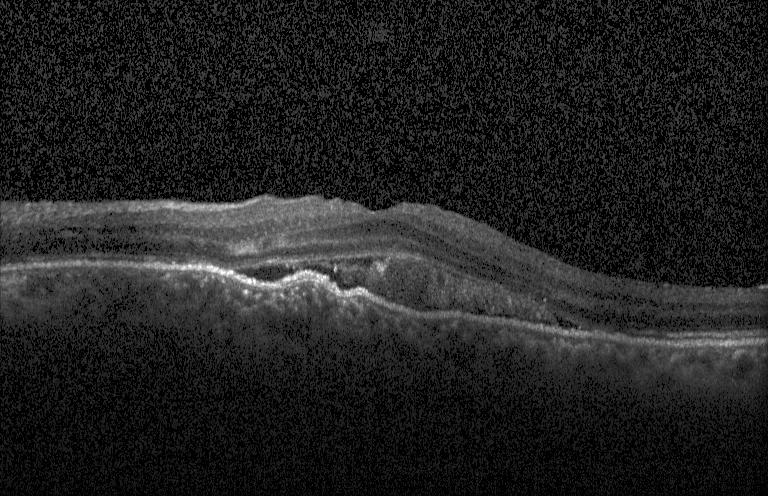
This B-scan demonstrates a choroidal neovascular membrane.